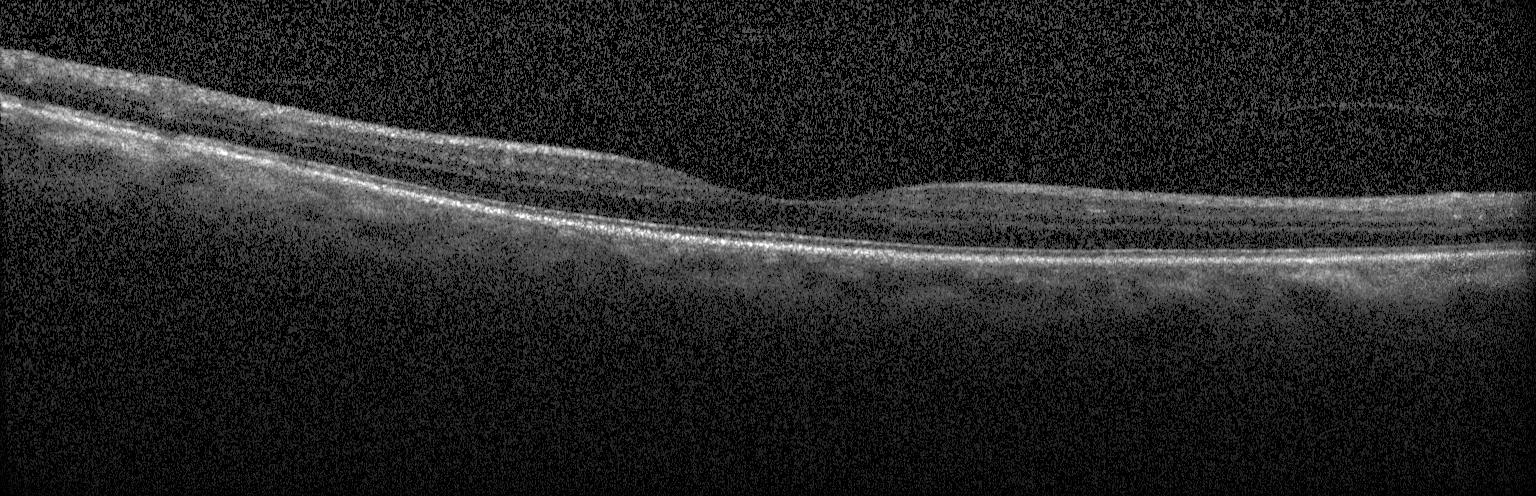

The scan shows no CNV, no DME, and no drusen.